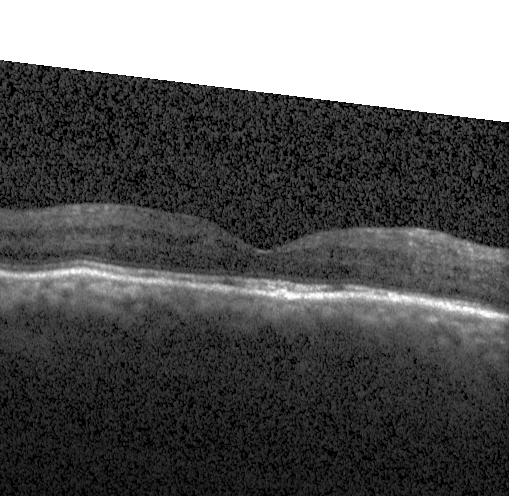

Macular OCT: no evidence of CNV, DME, or drusen.